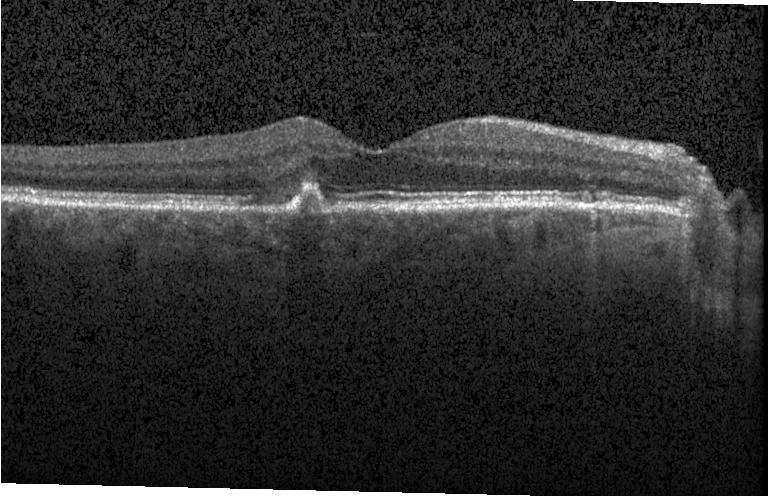 OCT line scan, Heidelberg Spectralis OCT system, macular scan.
Impression: a choroidal neovascular membrane.